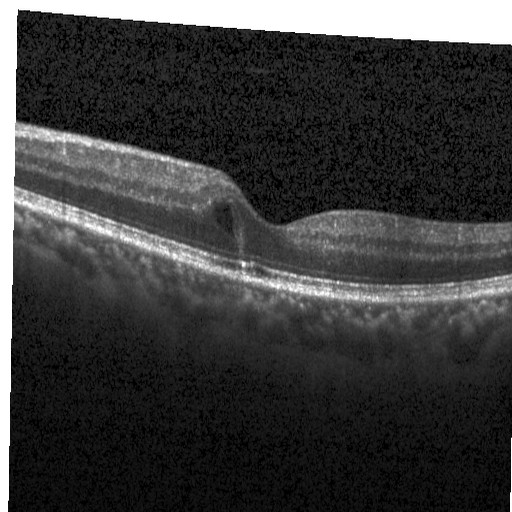 OCT B-scan, spectral-domain OCT, acquired on a Heidelberg Spectralis, centered on the fovea
Finding: diabetic macular edema.